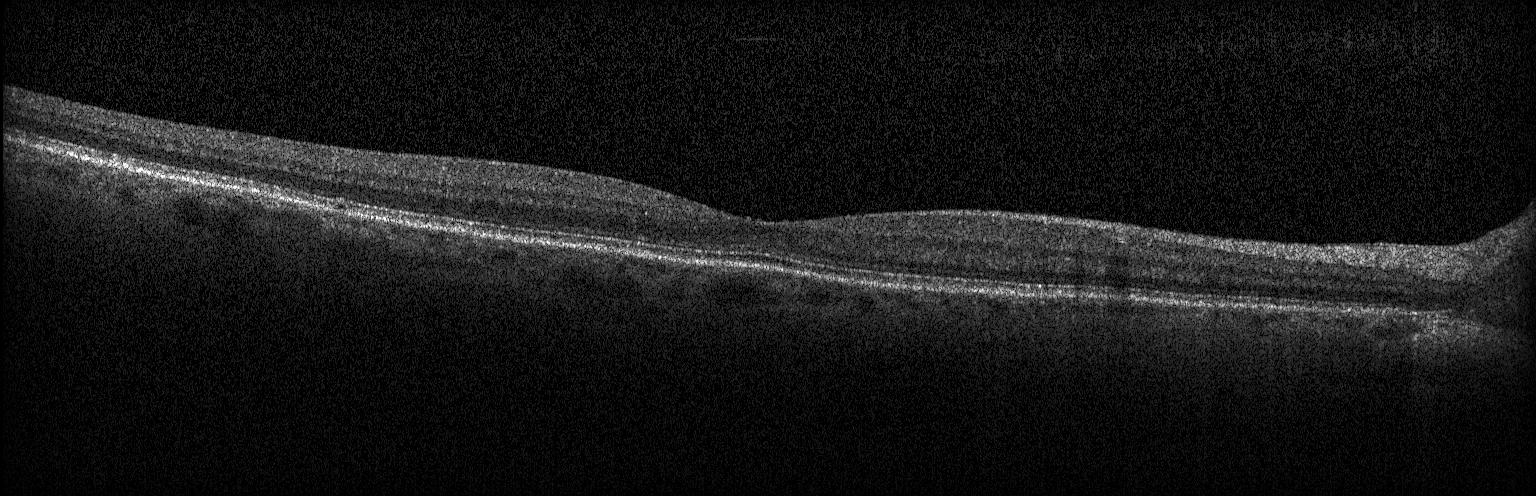

OCT finding: no evidence of choroidal neovascularization, diabetic macular edema, or drusen.